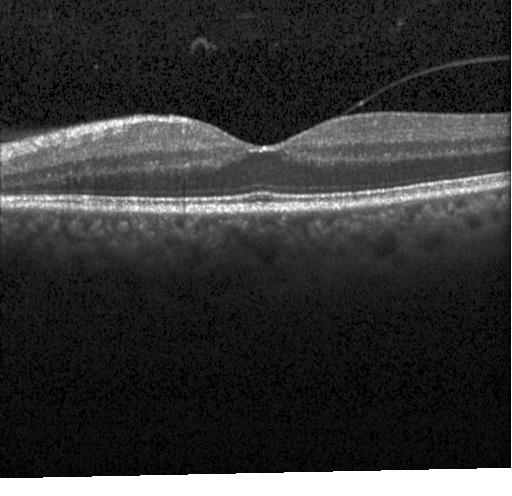 Spectral-domain OCT. Retinal OCT B-scan.
Finding: no evidence of CNV, DME, or drusen.